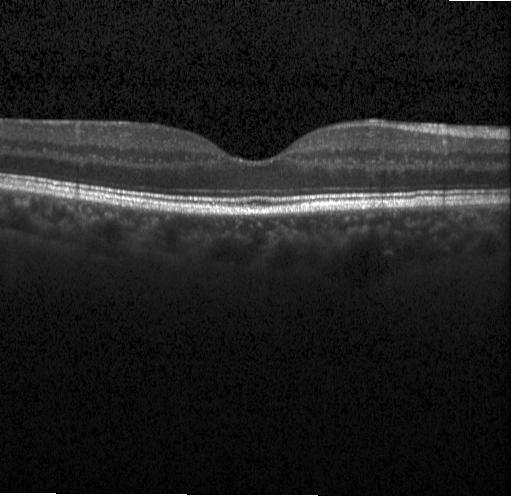
The scan shows no evidence of choroidal neovascularization, diabetic macular edema, or drusen.